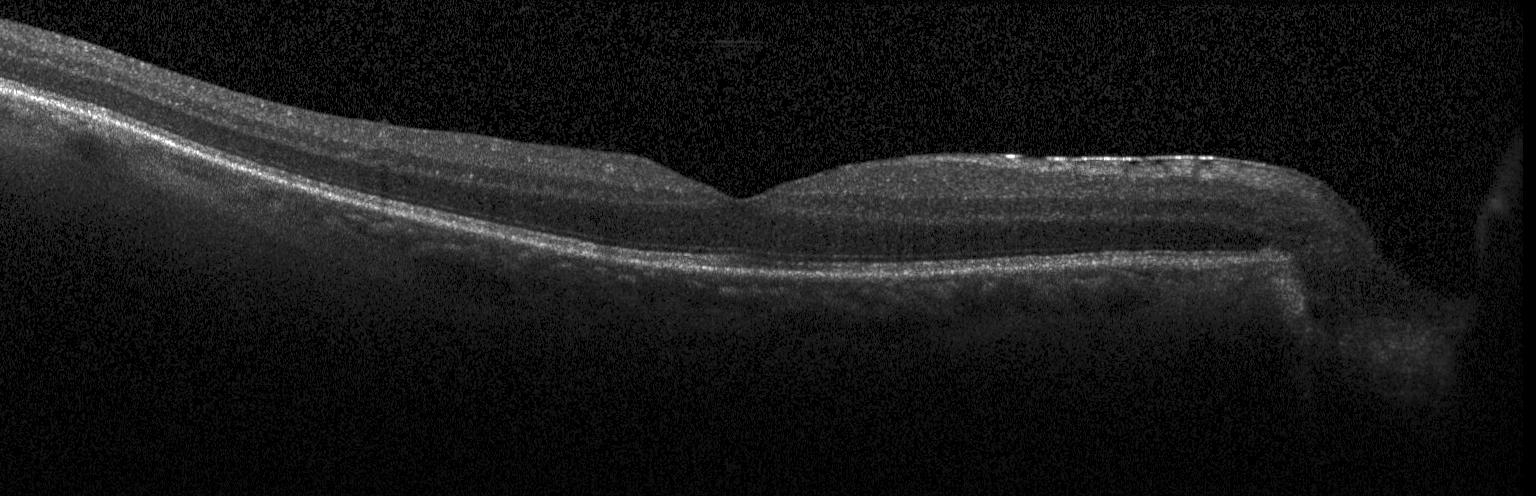
Retinal OCT cross-section showing no choroidal neovascularization, no diabetic macular edema, and no drusen.